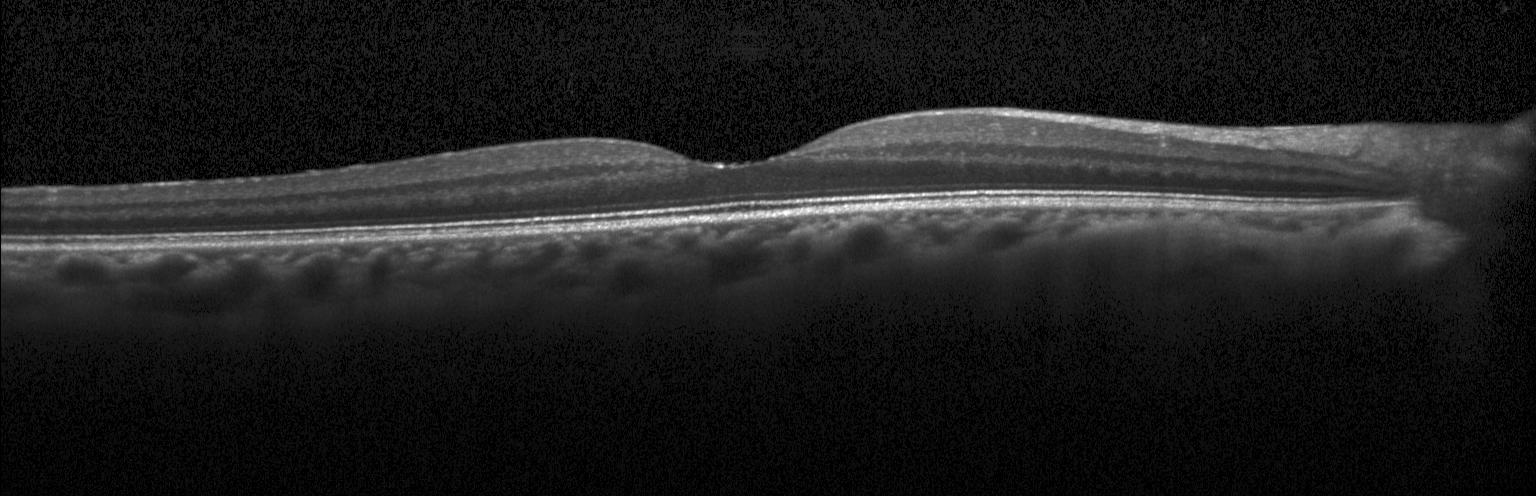 Centered on the fovea; optical coherence tomography B-scan; Heidelberg Spectralis OCT system; spectral-domain OCT.
Macular OCT: no evidence of CNV, DME, or drusen.